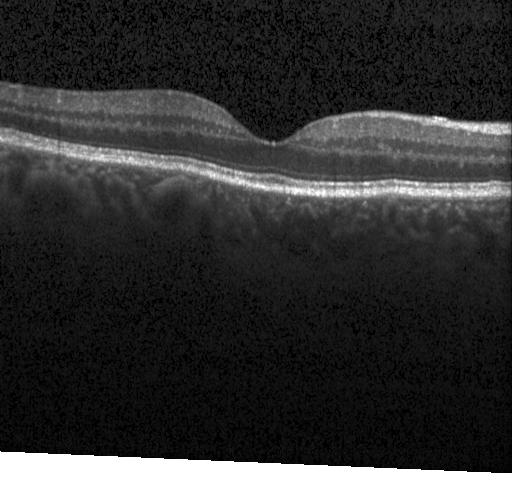

Centered on the fovea · retinal OCT B-scan · spectral-domain optical coherence tomography.
Macular OCT: no CNV, DME, or drusen.